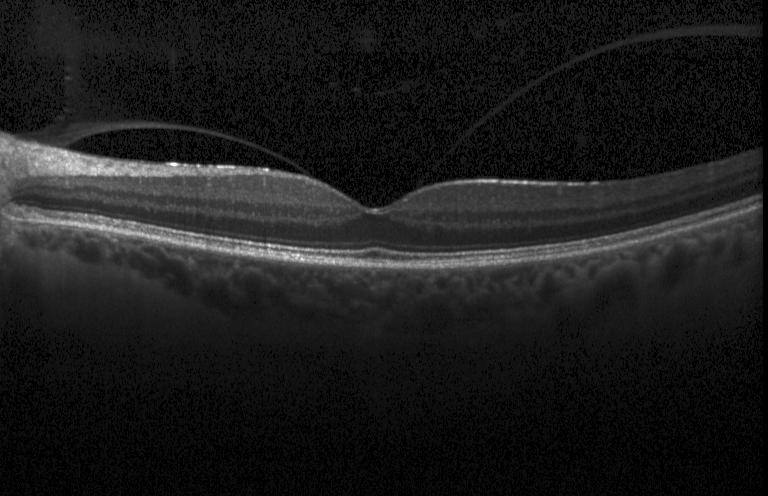
Retinal OCT B-scan, spectral-domain optical coherence tomography, Heidelberg Spectralis, through the macula.
Dx: no CNV, DME, or drusen.